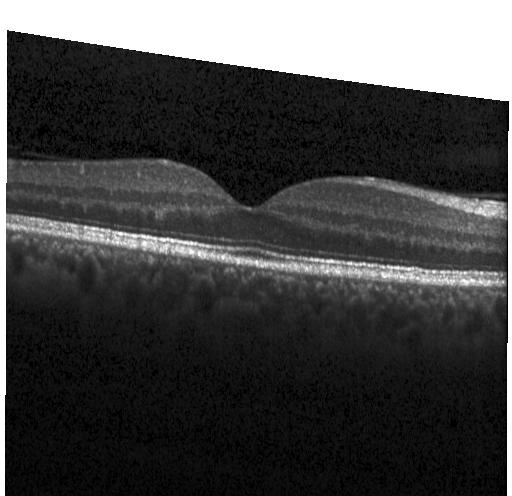

Macular OCT demonstrating no choroidal neovascularization, diabetic macular edema, or drusen.